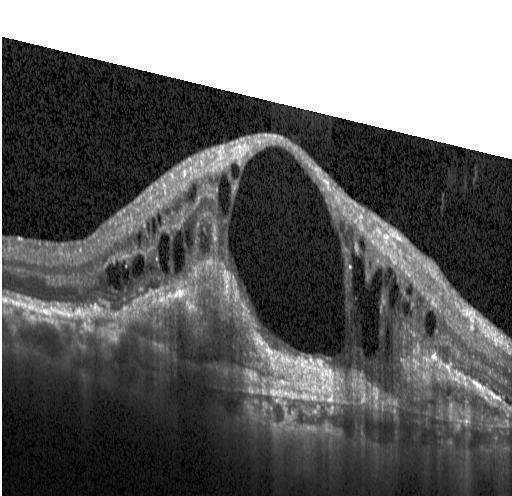
Impression: a choroidal neovascular membrane.